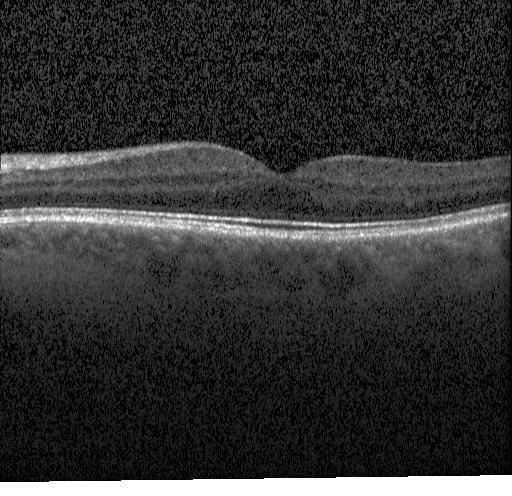
Retinal OCT cross-section.
This B-scan demonstrates no choroidal neovascularization, no diabetic macular edema, and no drusen.